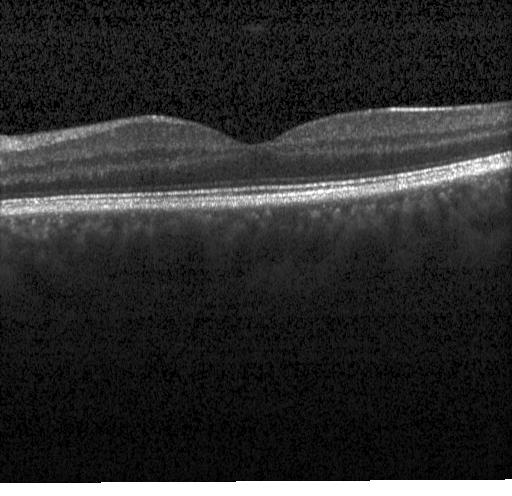

Impression: no evidence of CNV, DME, or drusen.